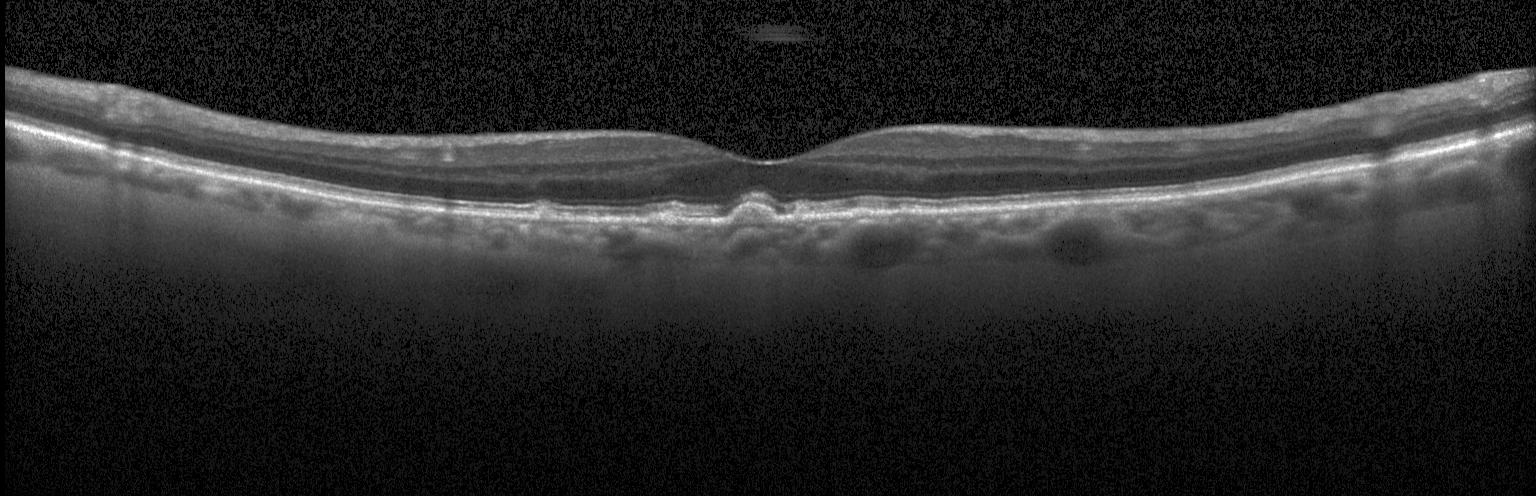

Retinal OCT B-scan
OCT finding: multiple drusen.